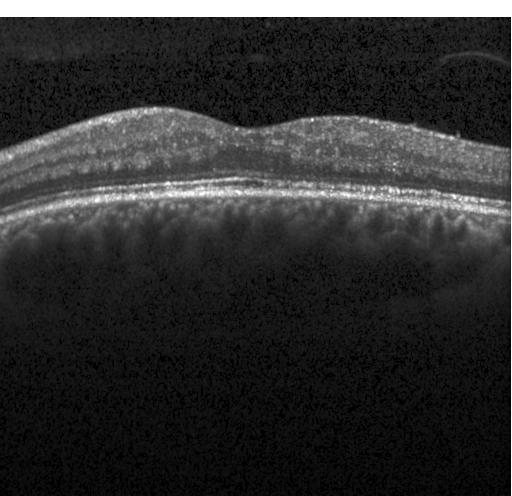 Retinal OCT B-scan. Impression: no evidence of choroidal neovascularization, diabetic macular edema, or drusen.